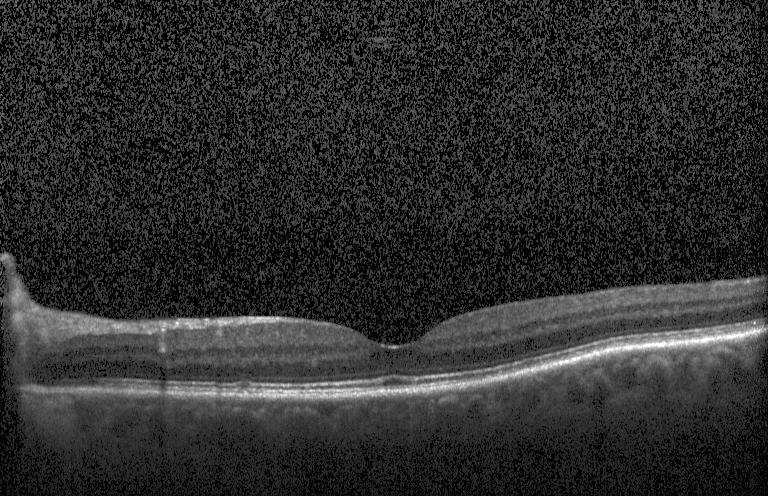 OCT B-scan, instrument: Heidelberg Spectralis, horizontal scan through the fovea — Macular OCT: neither CNV, DME, nor drusen.